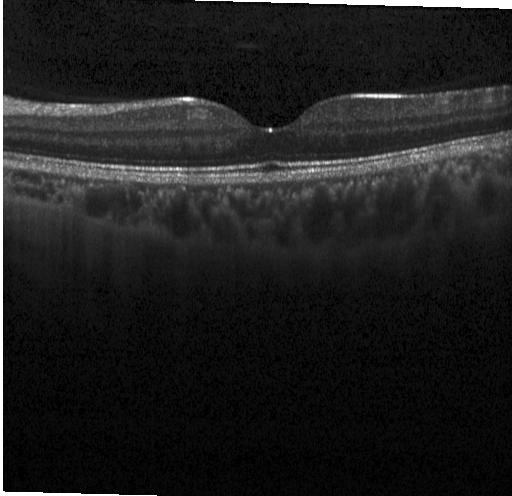

Diagnosis: neither choroidal neovascularization, diabetic macular edema, nor drusen.